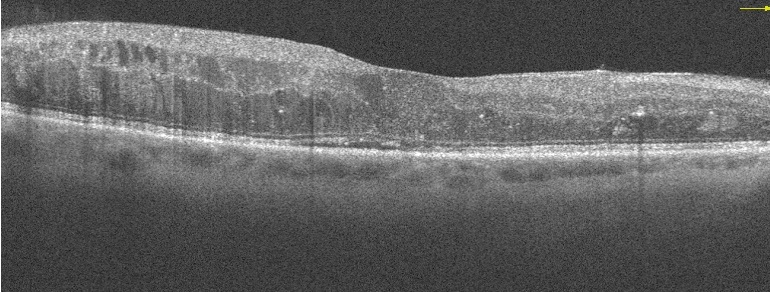 Diagnosis: diabetic macular edema (DME).